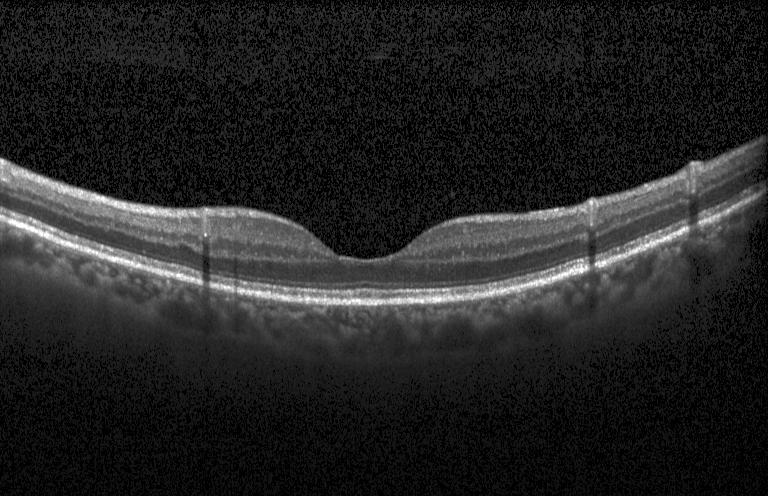
Diagnosis: no choroidal neovascularization, diabetic macular edema, or drusen.